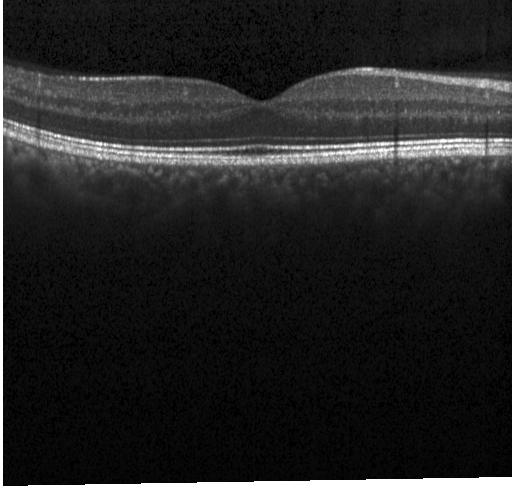

Assessment: neither choroidal neovascularization, diabetic macular edema, nor drusen.